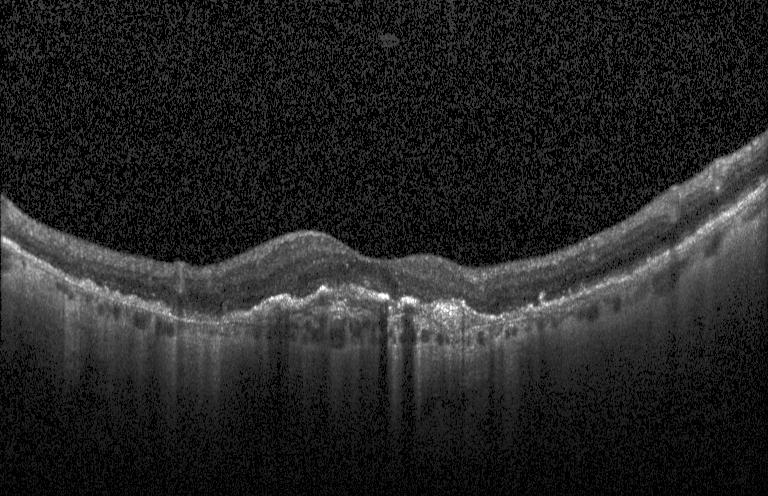 Impression: a choroidal neovascular membrane.